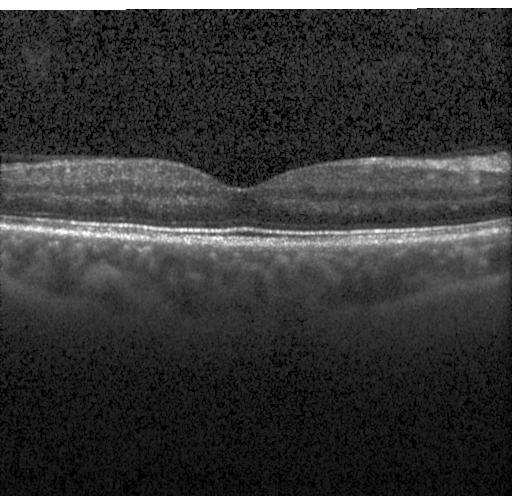 Retinal OCT B-scan.
Diagnosis: no evidence of choroidal neovascularization, diabetic macular edema, or drusen.